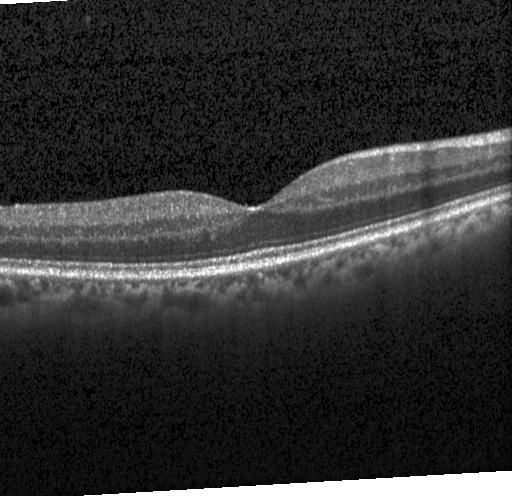 OCT B-scan showing neither choroidal neovascularization, diabetic macular edema, nor drusen.